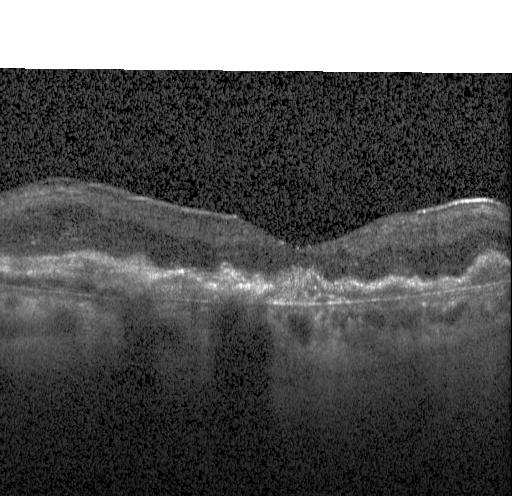 The scan shows choroidal neovascularization (CNV).